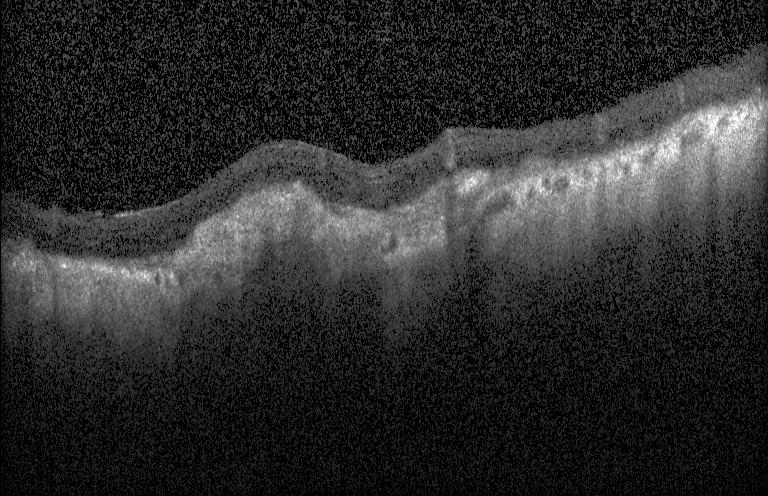
The scan shows choroidal neovascularization.